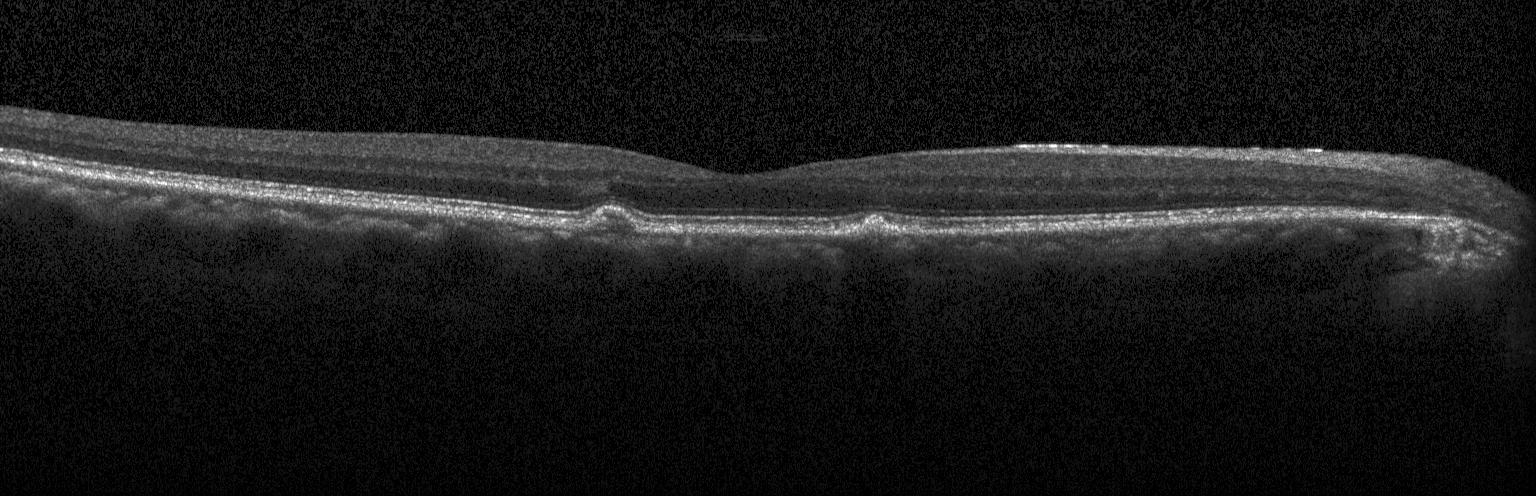
OCT line scan
The scan shows sub-RPE drusenoid deposits.